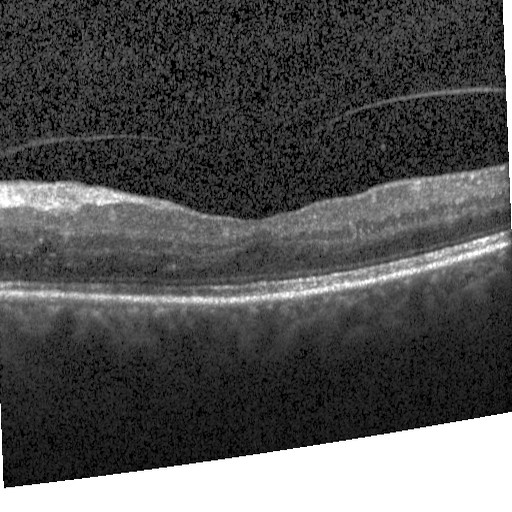
This B-scan demonstrates DME.